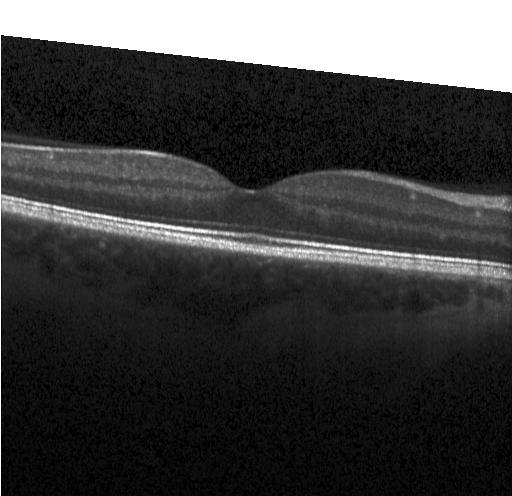 Spectral-domain optical coherence tomography, OCT B-scan. OCT finding: no evidence of choroidal neovascularization, diabetic macular edema, or drusen.